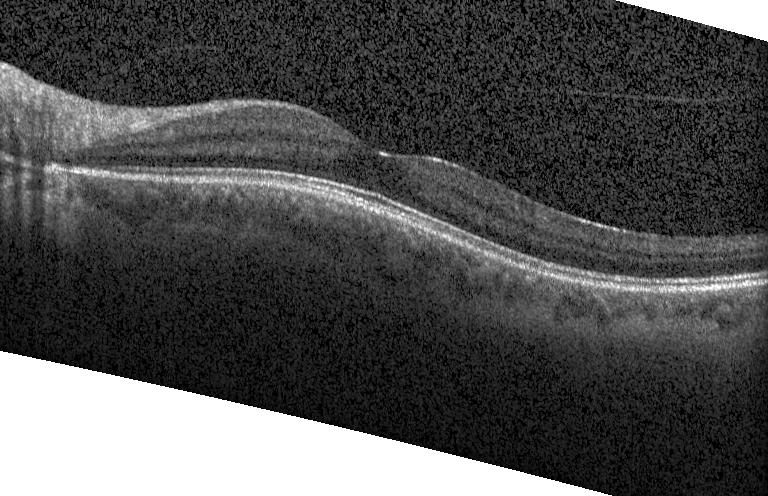 OCT B-scan, Heidelberg Spectralis, SD-OCT, macular scan. Diagnosis: no evidence of choroidal neovascularization, diabetic macular edema, or drusen.